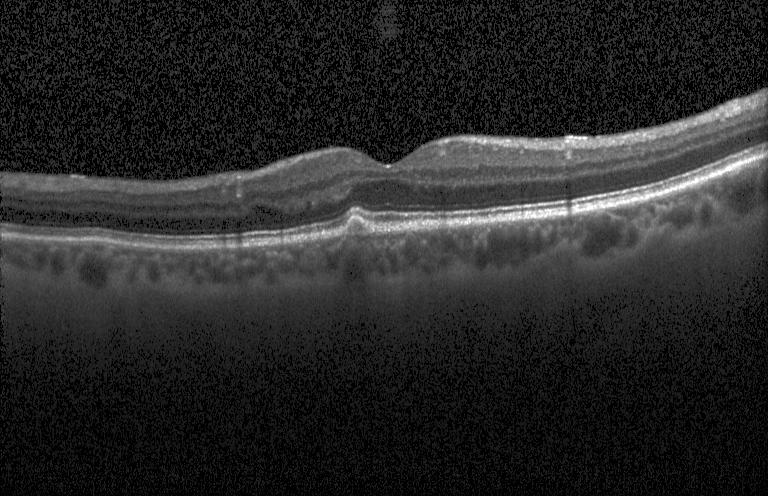

Macular OCT: drusen.